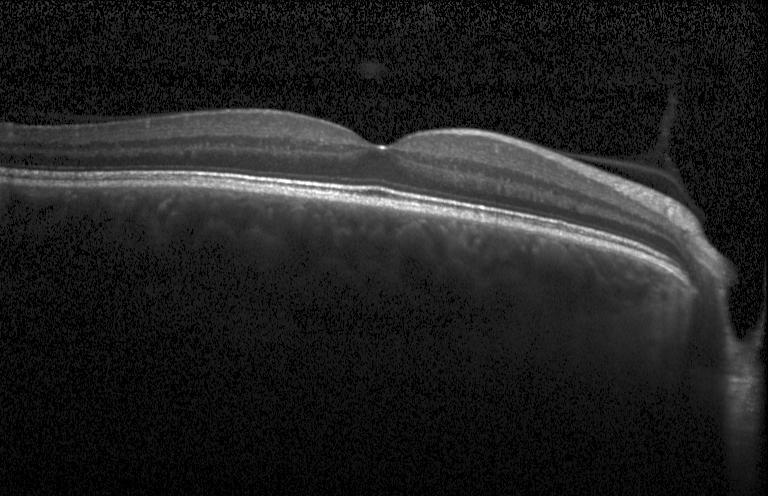
Retinal OCT cross-section showing neither CNV, DME, nor drusen.